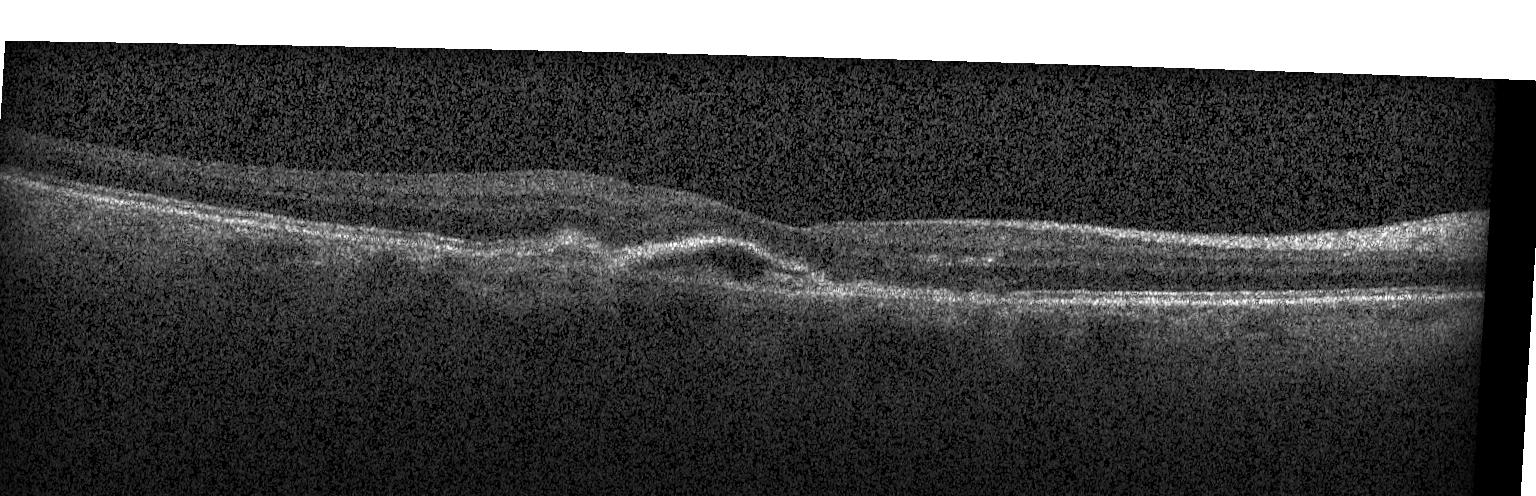 OCT B-scan. Finding: CNV.